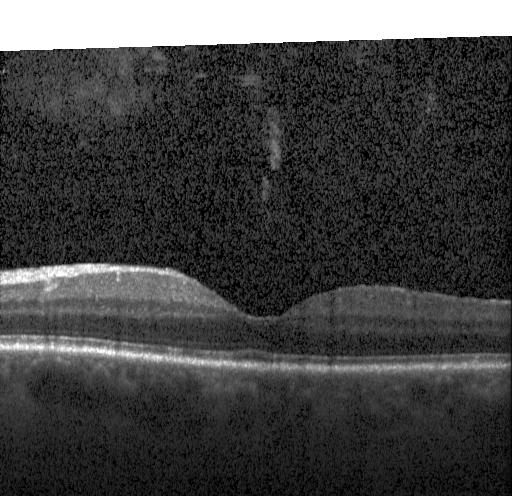

Horizontal scan through the fovea; retinal OCT B-scan; instrument: Heidelberg Spectralis; spectral-domain optical coherence tomography.
Macular OCT: no CNV, no DME, and no drusen.